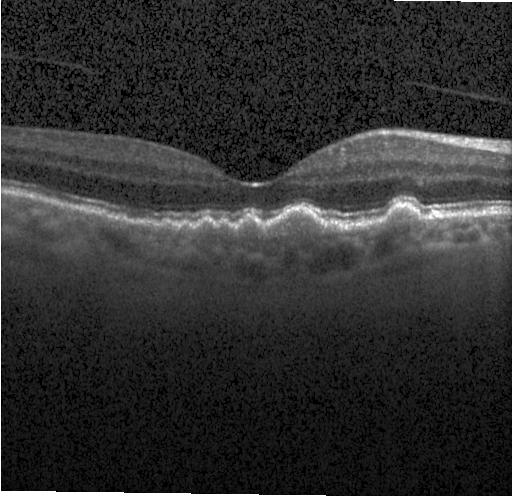
Finding: drusen.